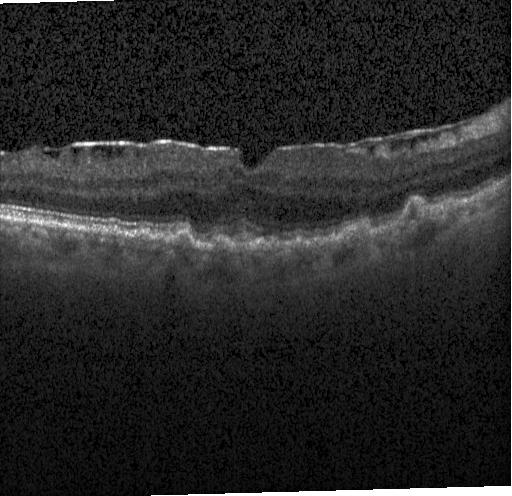 Multiple drusen.